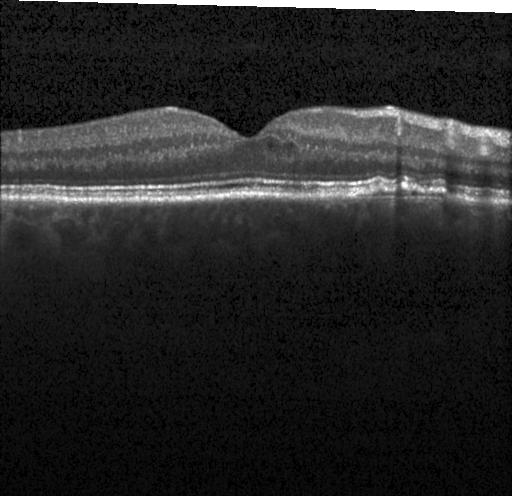
Optical coherence tomography B-scan, horizontal scan through the fovea, instrument: Heidelberg Spectralis.
Macular OCT: a choroidal neovascular membrane.